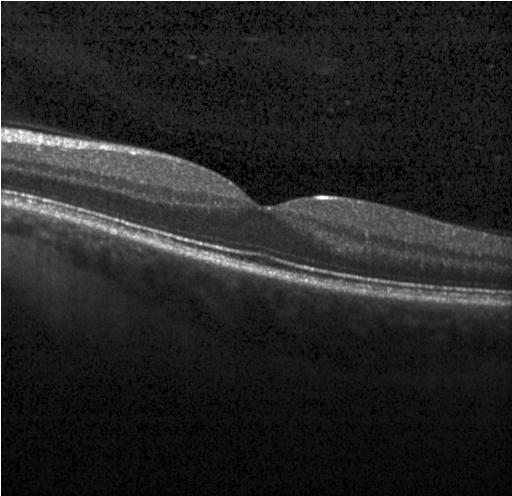 Heidelberg Spectralis. Retinal OCT B-scan. Macular scan. OCT finding: neither choroidal neovascularization, diabetic macular edema, nor drusen.